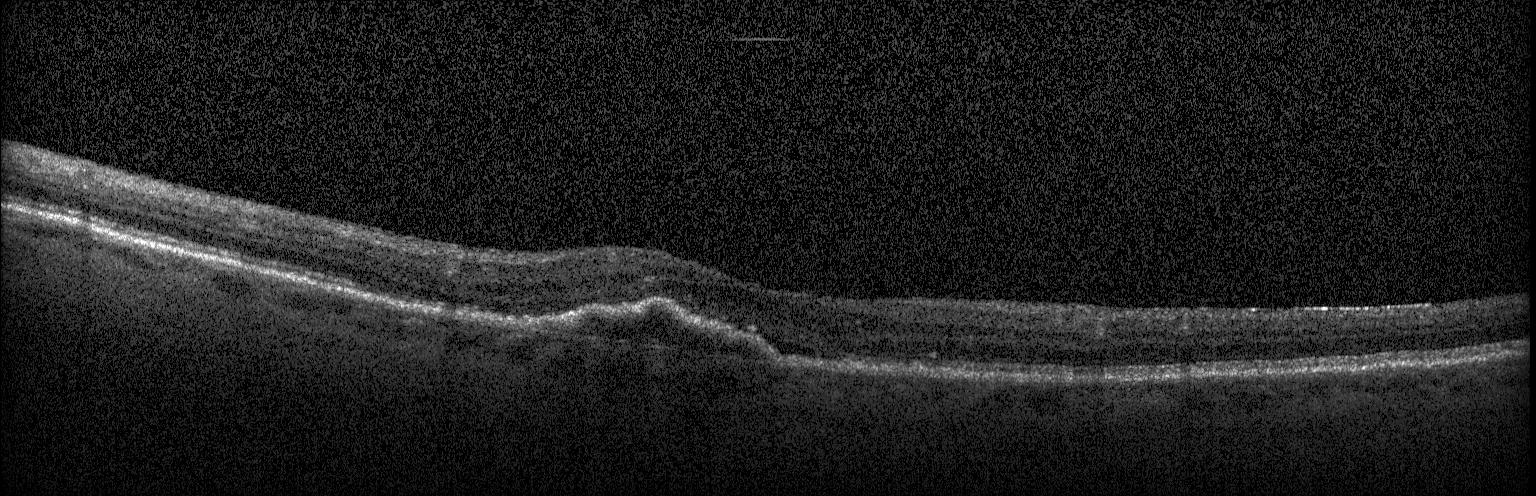

Spectral-domain optical coherence tomography. Retinal OCT B-scan
Finding: a choroidal neovascular membrane.